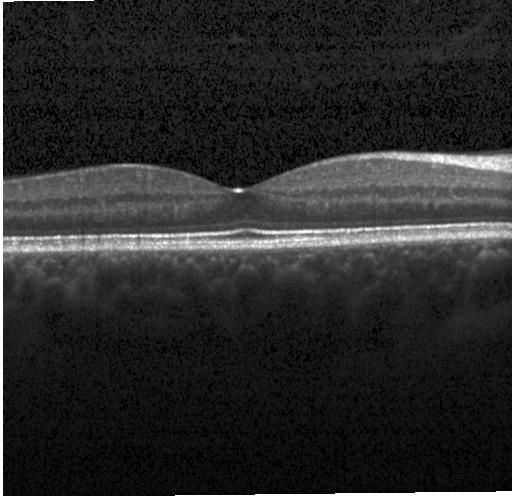

The scan shows no choroidal neovascularization, diabetic macular edema, or drusen.